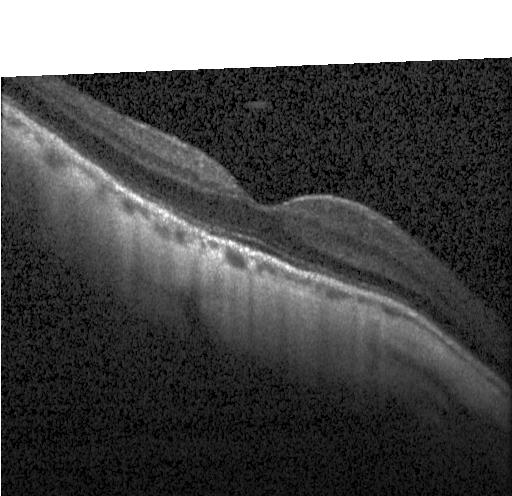

Acquired on a Heidelberg Spectralis, horizontal scan through the fovea, retinal OCT B-scan. Diagnosis: neither choroidal neovascularization, diabetic macular edema, nor drusen.